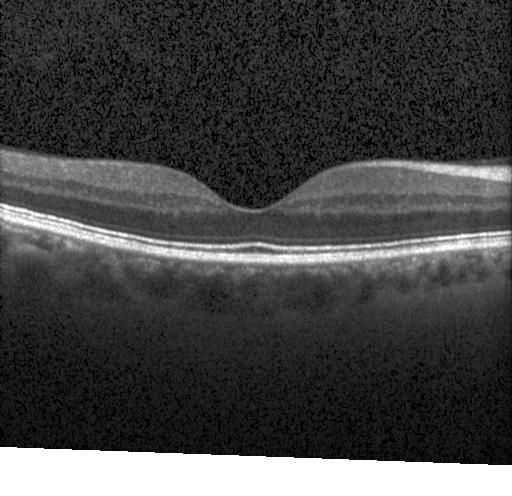
Fovea-centered · spectral-domain optical coherence tomography · optical coherence tomography scan.
Diagnosis: no choroidal neovascularization, no diabetic macular edema, and no drusen.